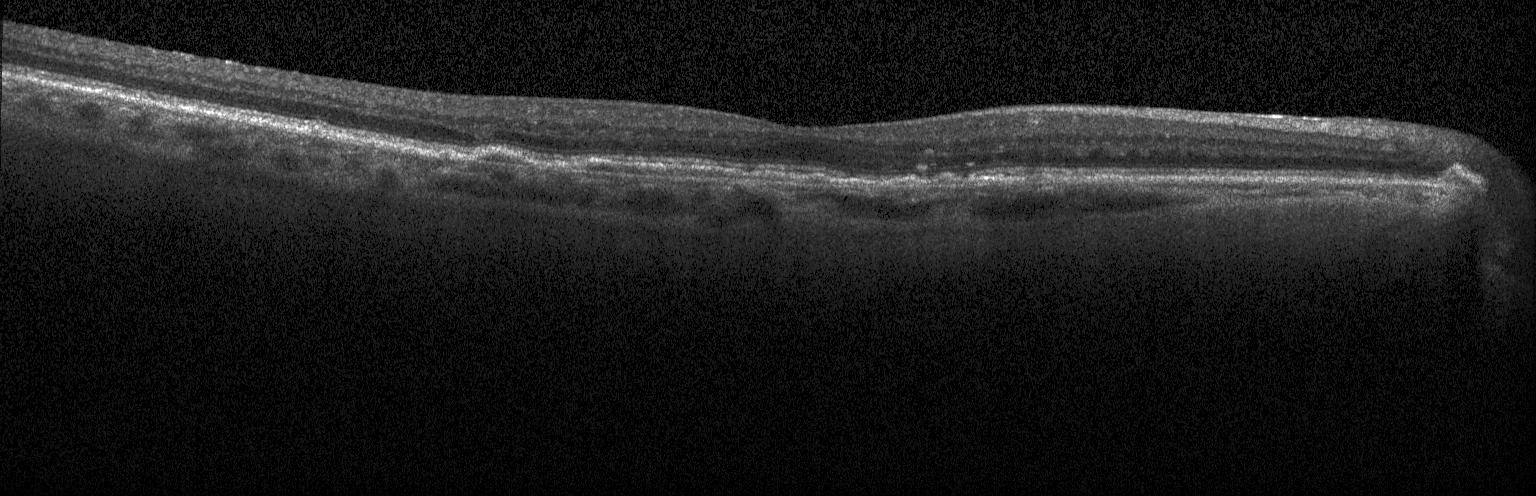

OCT line scan, fovea-centered
Diagnosis: choroidal neovascularization.